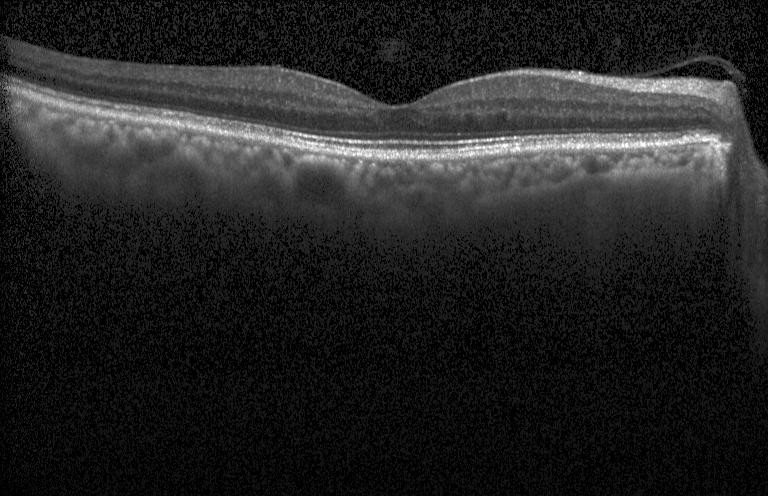 Macular scan; optical coherence tomography B-scan; Heidelberg Spectralis OCT system; spectral-domain OCT. Finding: no choroidal neovascularization, diabetic macular edema, or drusen.